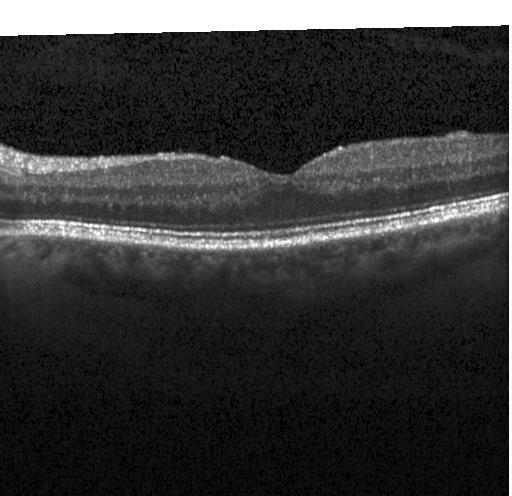 Heidelberg Spectralis; retinal OCT B-scan; fovea-centered
Finding: no CNV, no DME, and no drusen.